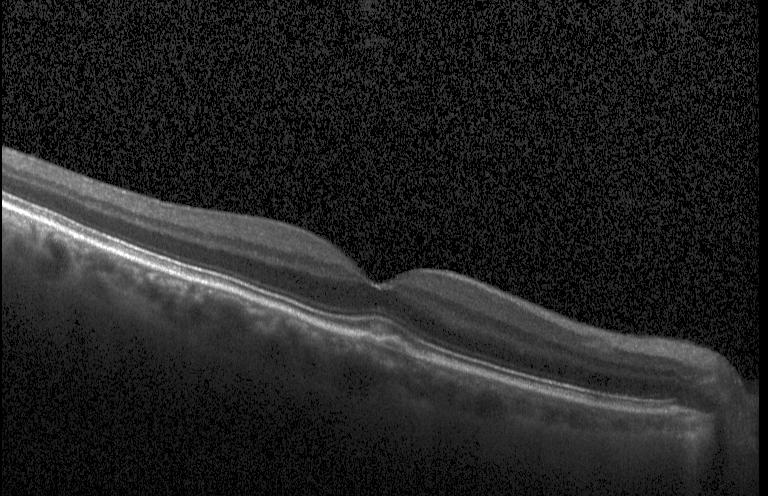 Retinal OCT cross-section · fovea-centered. Assessment: a choroidal neovascular membrane.